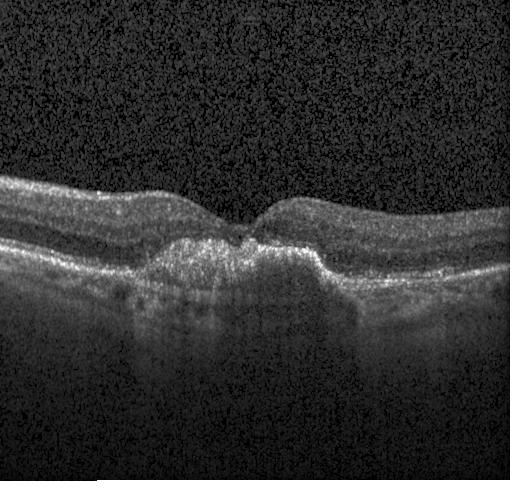 OCT line scan
OCT finding: choroidal neovascularization.